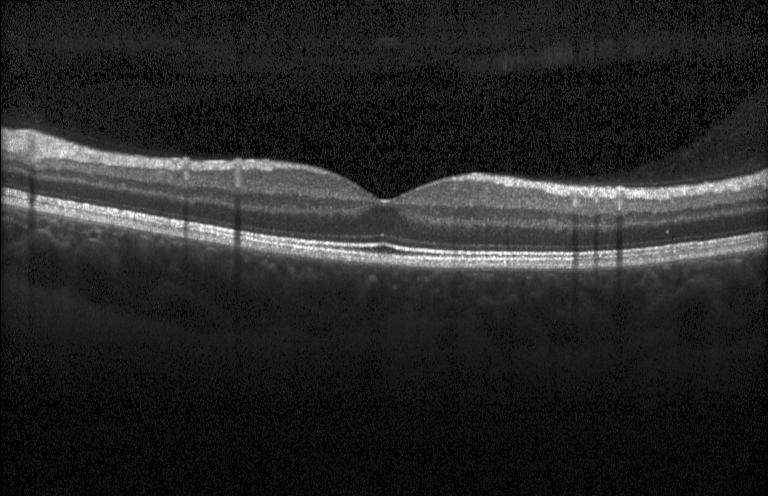
Retinal OCT cross-section · acquired on a Heidelberg Spectralis.
Diagnosis: no CNV, no DME, and no drusen.